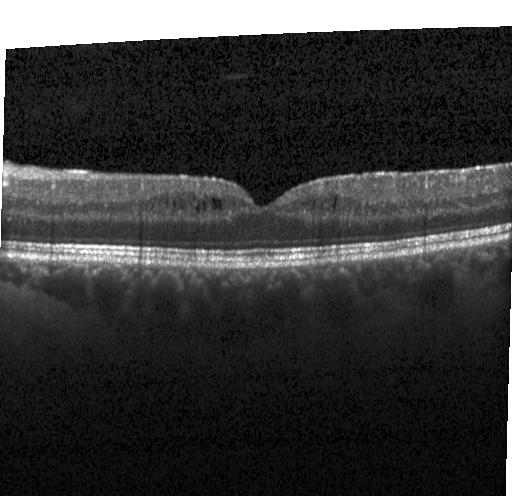
Assessment: diabetic macular edema (DME).